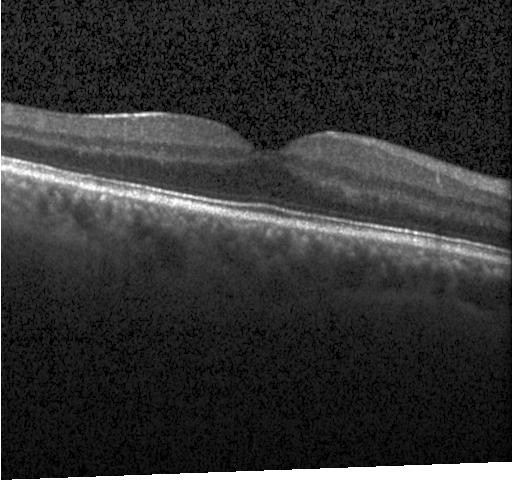
OCT finding: no choroidal neovascularization, no diabetic macular edema, and no drusen.